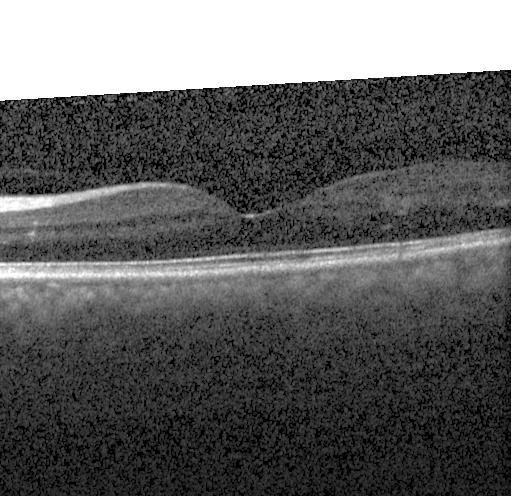
Optical coherence tomography B-scan · spectral-domain optical coherence tomography · fovea-centered.
The scan shows neither CNV, DME, nor drusen.